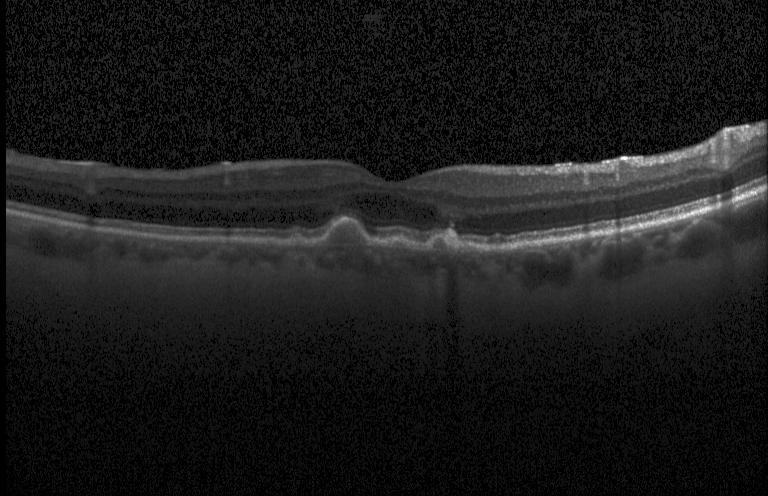 Fovea-centered. SD-OCT. OCT line scan
Assessment: multiple drusen.